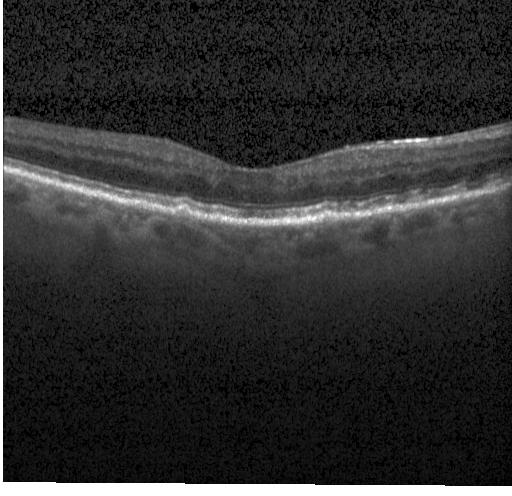 Spectral-domain optical coherence tomography · retinal OCT cross-section. Dx: sub-RPE drusenoid deposits.